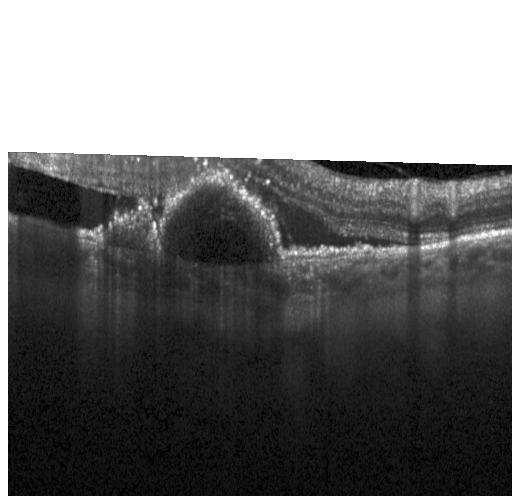
OCT scan showing choroidal neovascularization (CNV).